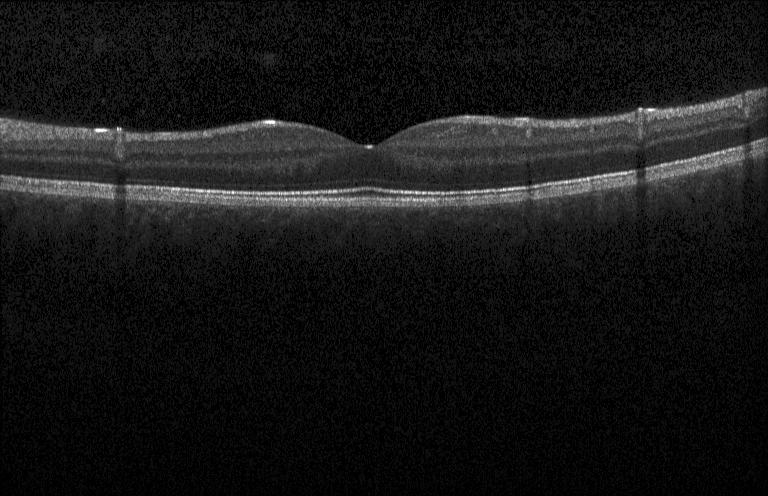
Retinal OCT cross-section, spectral-domain OCT, Heidelberg Spectralis, centered on the fovea. Dx: neither choroidal neovascularization, diabetic macular edema, nor drusen.